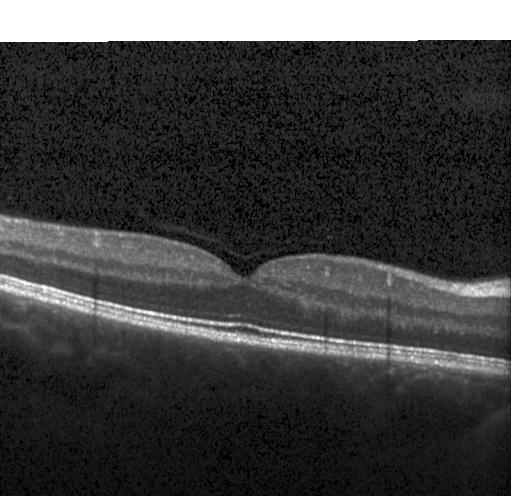
Impression: neither CNV, DME, nor drusen.